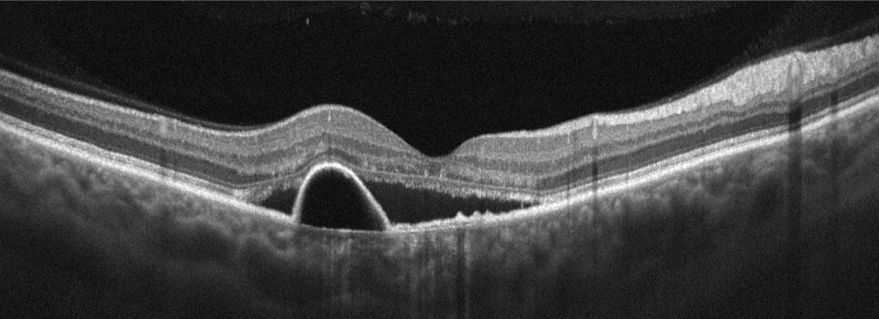

OCT line scan — OCT finding: AMD.